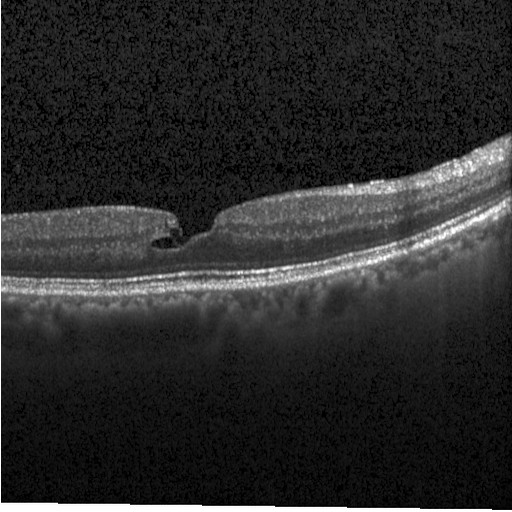 OCT B-scan · Heidelberg Spectralis · through the macula · SD-OCT.
Dx: diabetic macular edema.